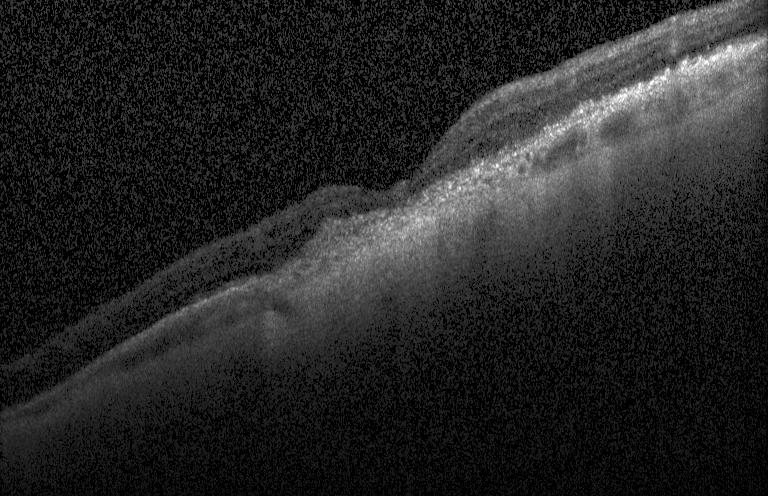
Dx: choroidal neovascularization.